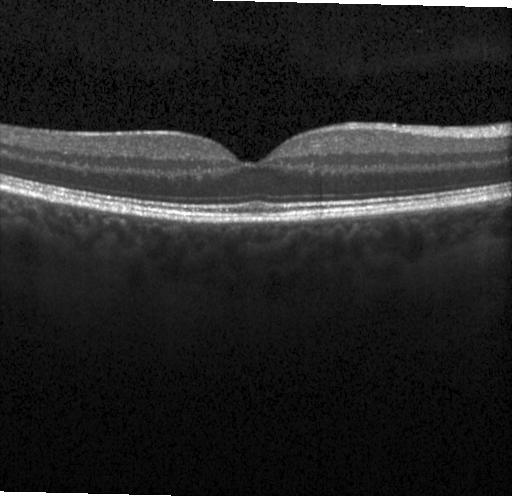
Dx: no choroidal neovascularization, diabetic macular edema, or drusen.